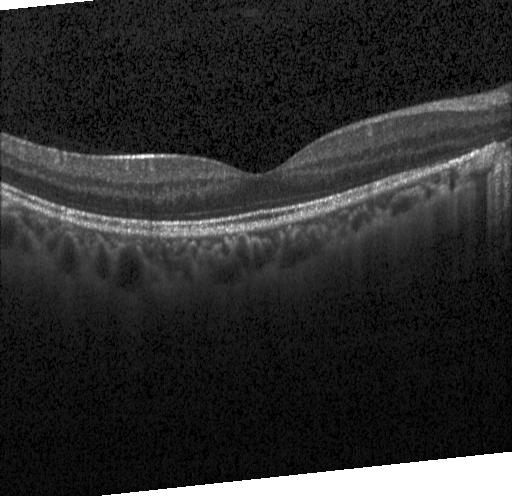 Retinal OCT cross-section, spectral-domain OCT
Finding: neither choroidal neovascularization, diabetic macular edema, nor drusen.